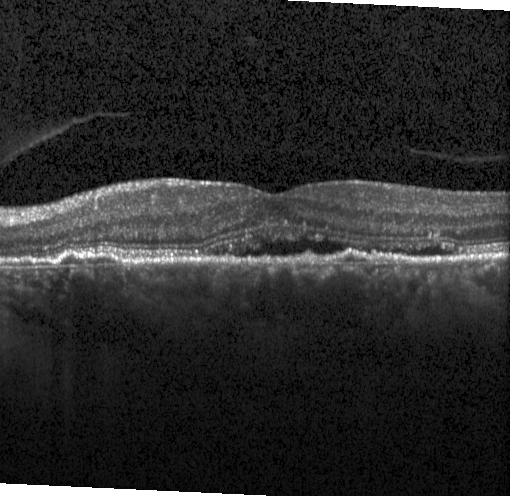 Assessment: a choroidal neovascular membrane.